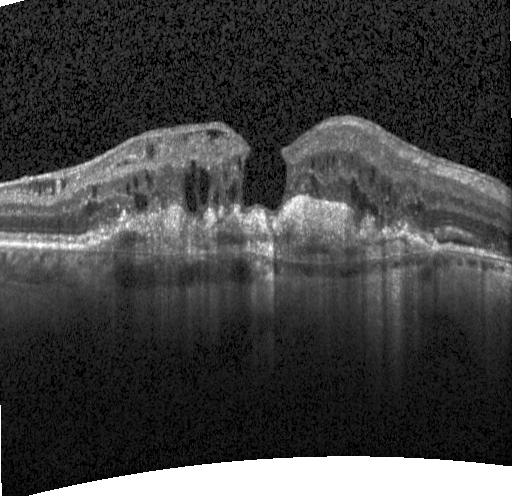

OCT line scan. Instrument: Heidelberg Spectralis. Finding: choroidal neovascularization (CNV).